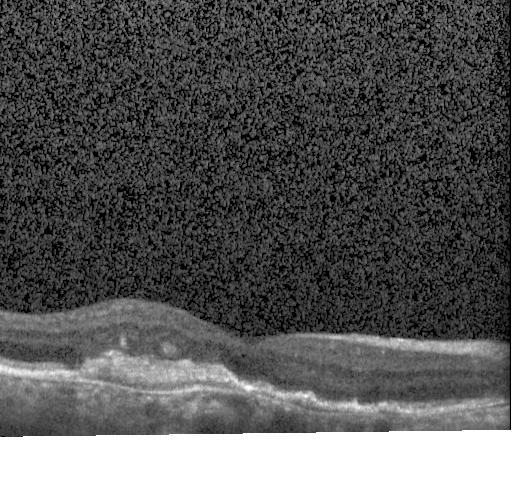

Centered on the fovea, acquired on a Heidelberg Spectralis, retinal OCT B-scan — Finding: CNV.